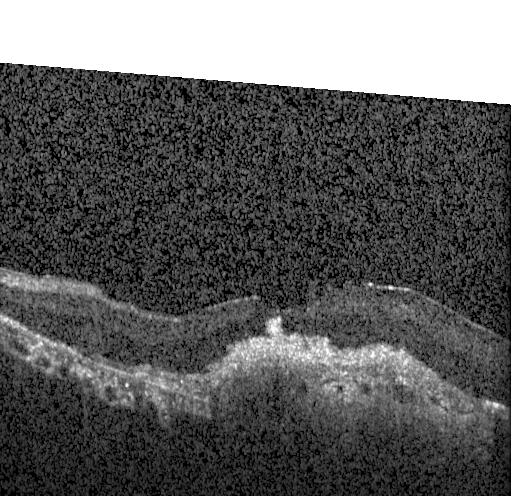 Centered on the fovea · optical coherence tomography scan
Dx: choroidal neovascularization (CNV).